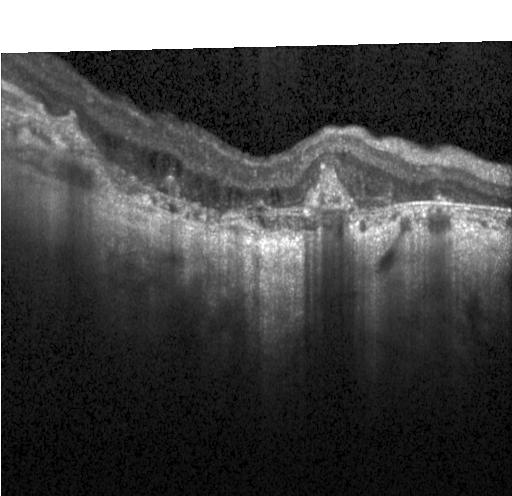

The scan shows CNV.